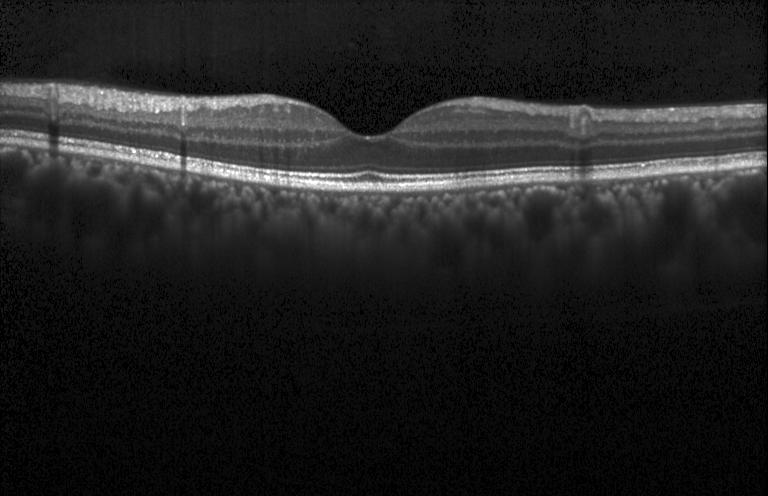
OCT scan showing no evidence of choroidal neovascularization, diabetic macular edema, or drusen.